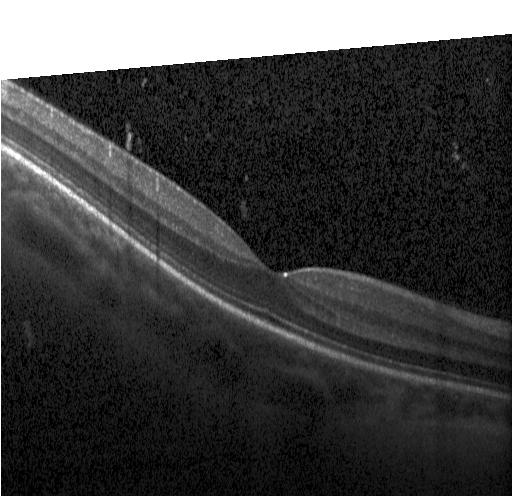
Assessment: neither choroidal neovascularization, diabetic macular edema, nor drusen.